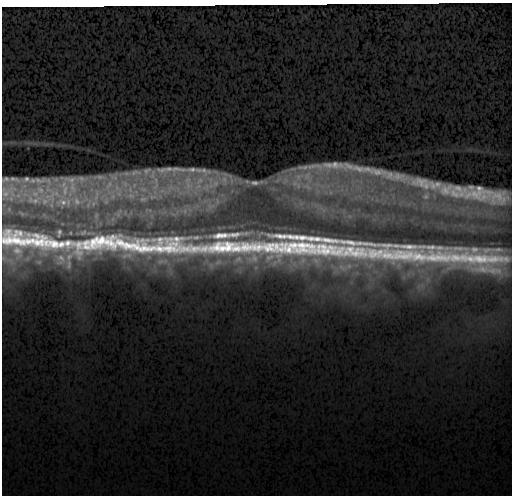 Macular OCT: CNV.